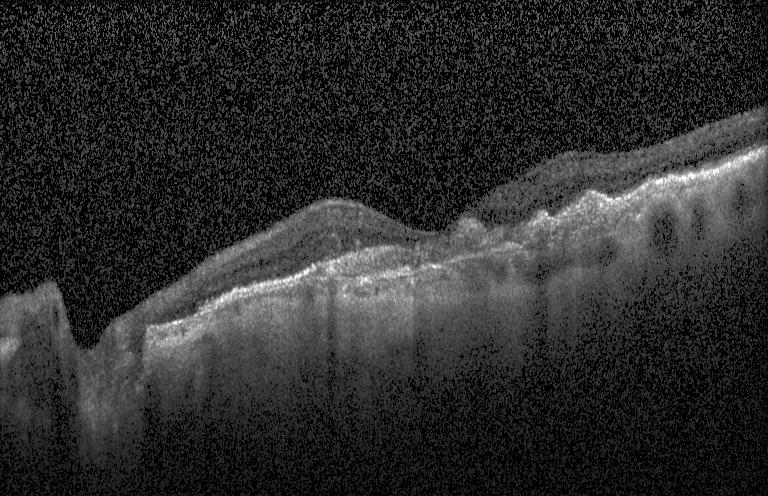
Retinal OCT cross-section showing choroidal neovascularization (CNV).